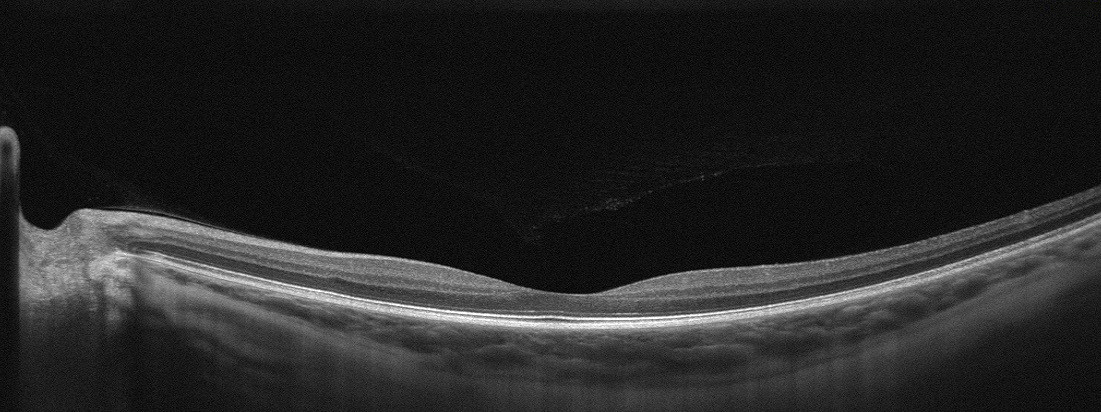

Instrument: Optovue Avanti RTVue XR, retinal OCT B-scan, fovea-centered
Dx: no evidence of AMD, DME, ERM, RAO, RVO, or VID.